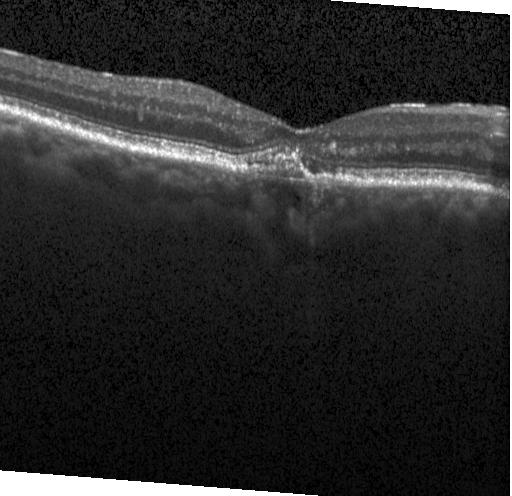 OCT finding: CNV.